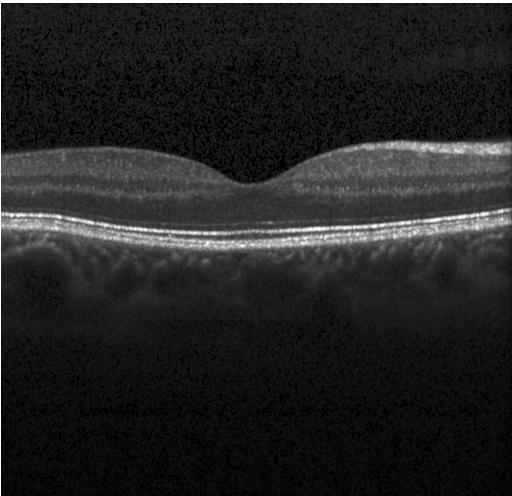

Retinal OCT cross-section.
Finding: no evidence of choroidal neovascularization, diabetic macular edema, or drusen.